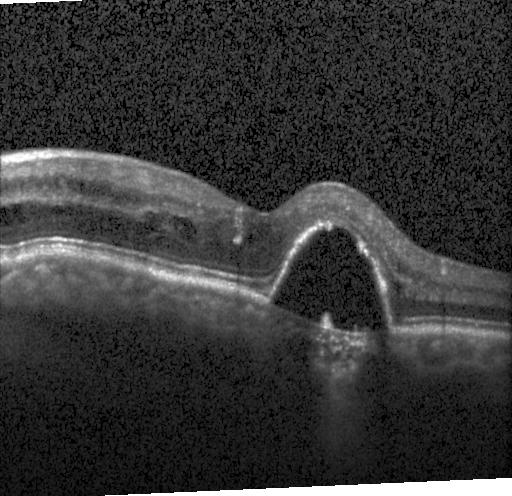
Choroidal neovascularization.